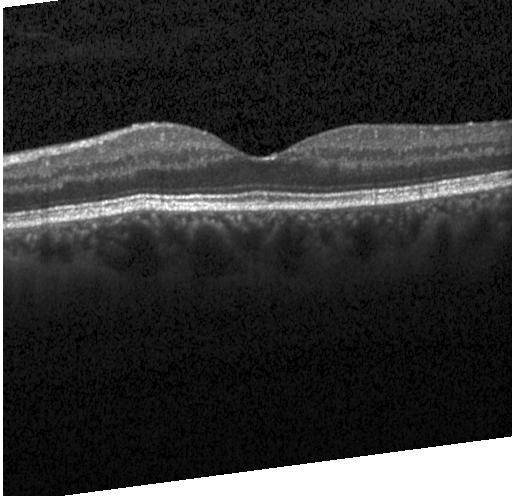 Centered on the fovea, OCT B-scan, SD-OCT — Impression: no evidence of CNV, DME, or drusen.